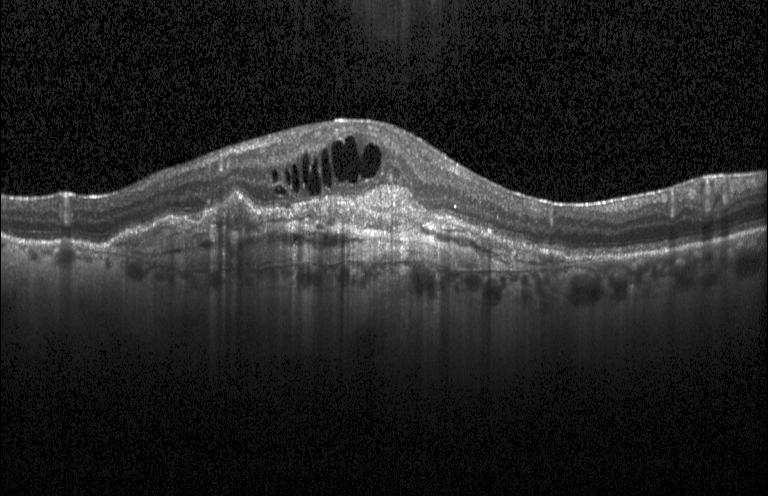

Macular scan; retinal OCT B-scan.
The scan shows a choroidal neovascular membrane.